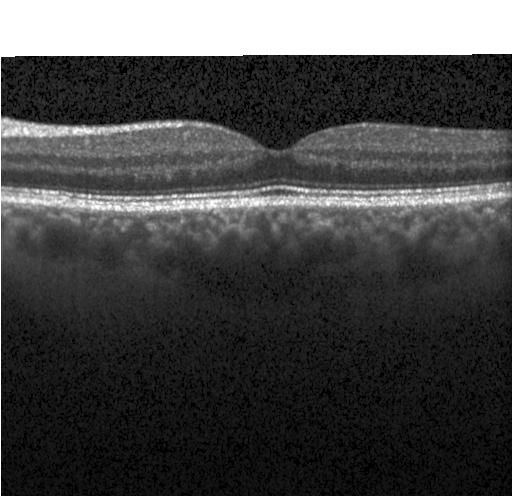

OCT B-scan showing no choroidal neovascularization, no diabetic macular edema, and no drusen.